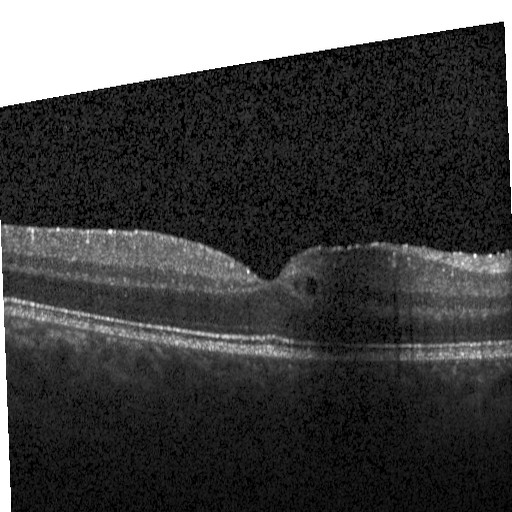
Fovea-centered. Retinal OCT cross-section. Acquired on a Heidelberg Spectralis. Spectral-domain optical coherence tomography.
Assessment: diabetic macular edema (DME).